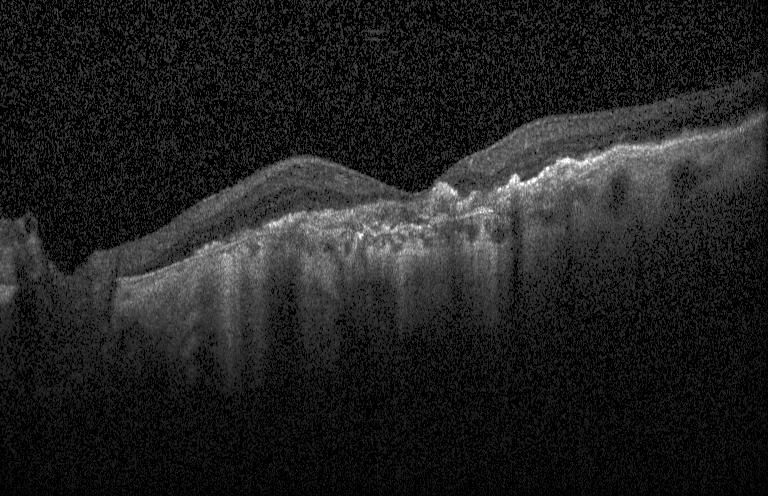
Spectral-domain OCT B-scan: CNV.